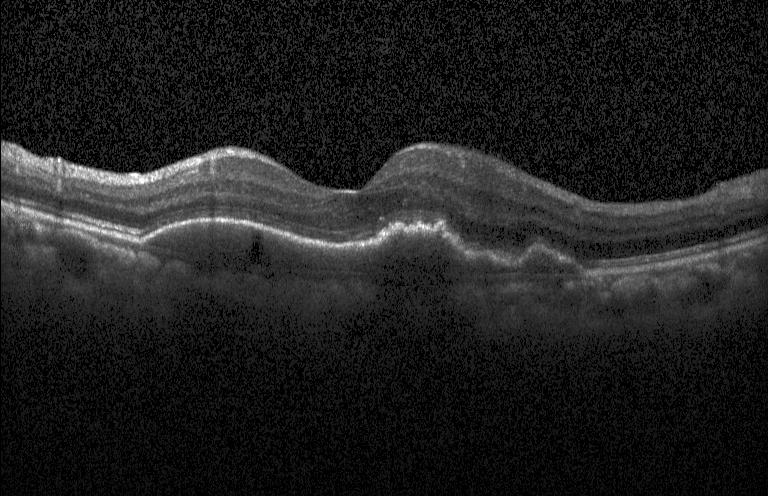
Acquired on a Heidelberg Spectralis. OCT line scan. This B-scan demonstrates a choroidal neovascular membrane.